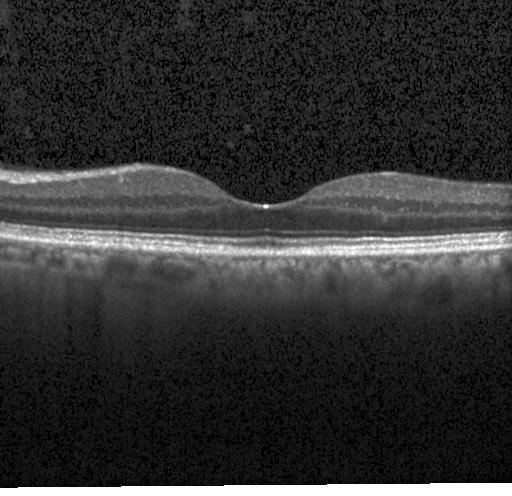 Horizontal scan through the fovea. Retinal OCT cross-section. Instrument: Heidelberg Spectralis. Diagnosis: no evidence of CNV, DME, or drusen.